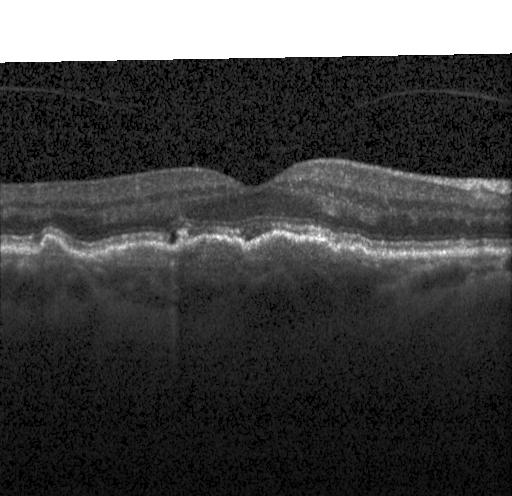

Optical coherence tomography scan.
Impression: a choroidal neovascular membrane.